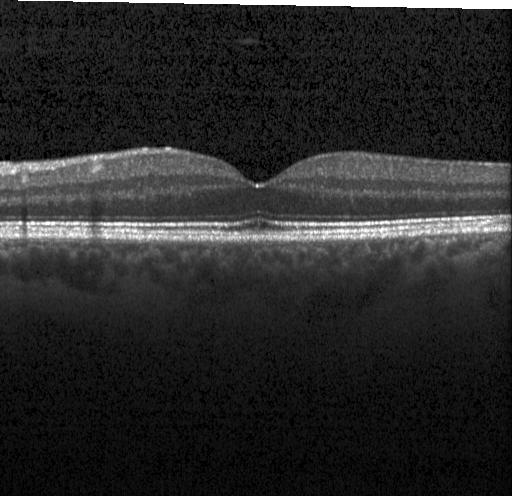

Impression: no choroidal neovascularization, no diabetic macular edema, and no drusen.